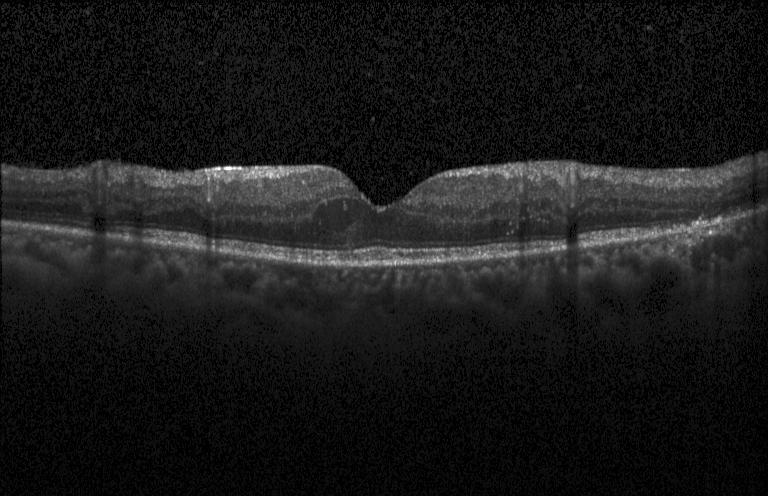

Assessment: diabetic macular edema.